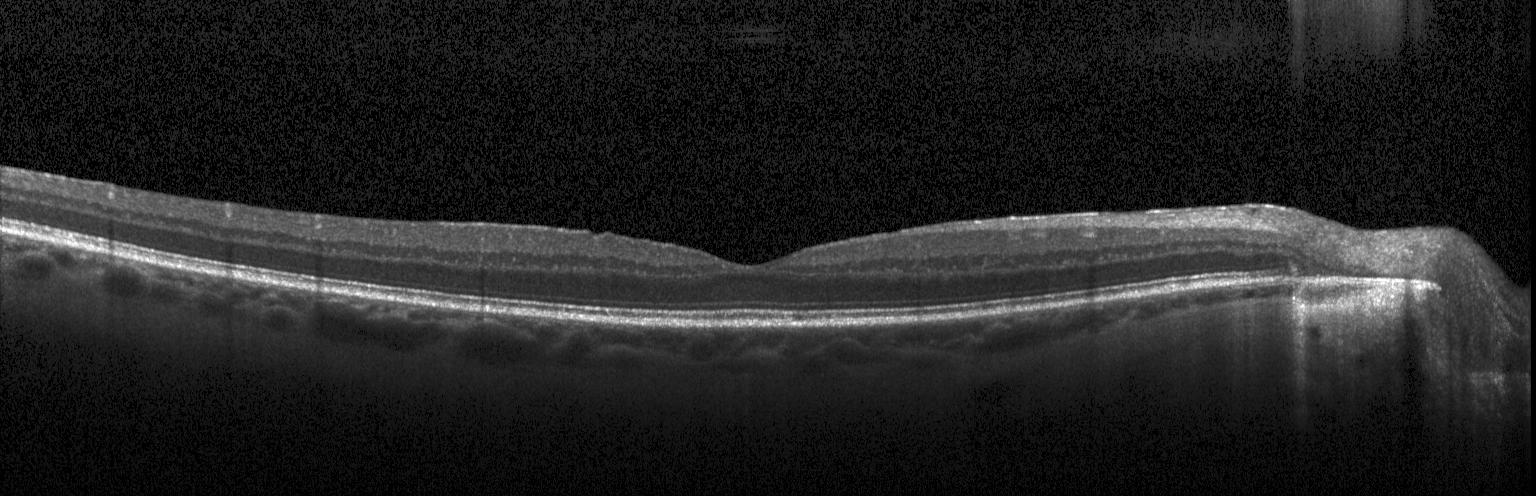
No choroidal neovascularization, diabetic macular edema, or drusen.